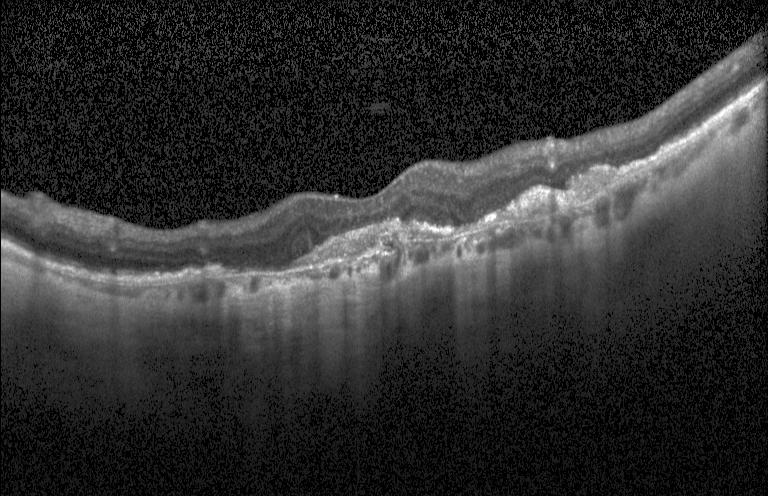
OCT finding: a choroidal neovascular membrane.